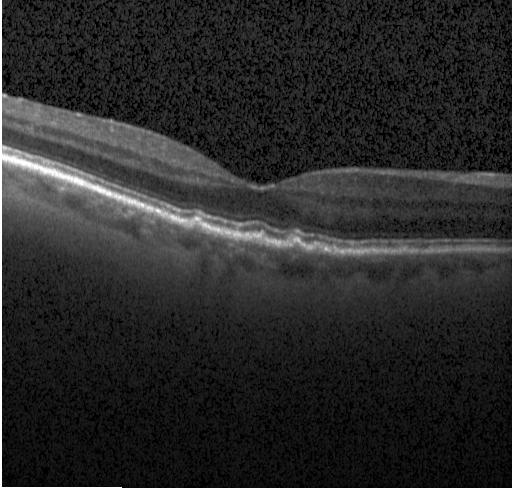

OCT line scan. Heidelberg Spectralis.
Dx: drusen.